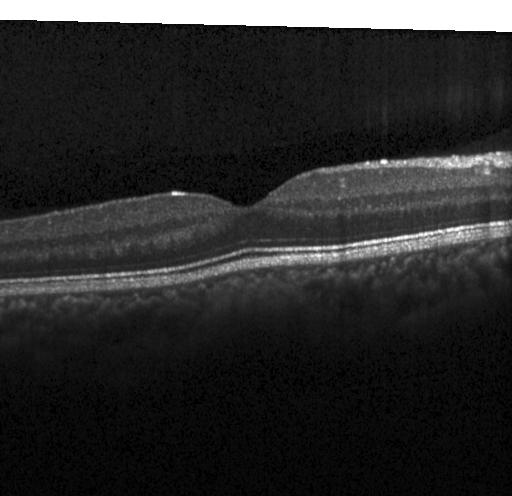 Spectral-domain OCT B-scan: neither choroidal neovascularization, diabetic macular edema, nor drusen.